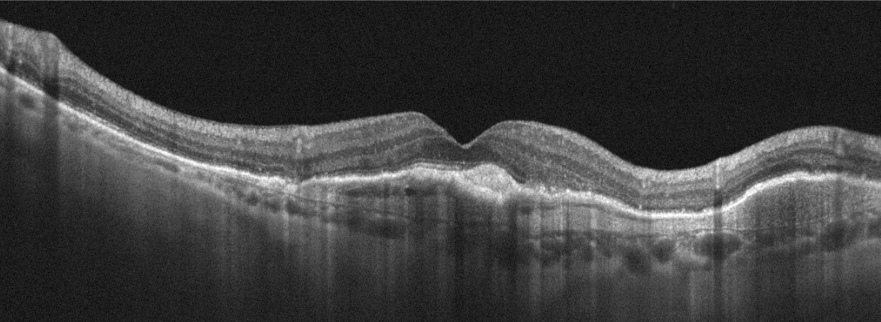

Through the macula; retinal OCT B-scan; acquired on an Optovue Avanti RTVue XR.
Impression: age-related macular degeneration.